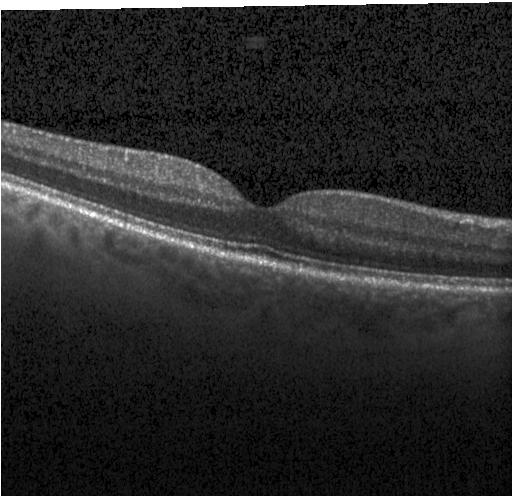 Optical coherence tomography B-scan. This B-scan demonstrates no CNV, no DME, and no drusen.